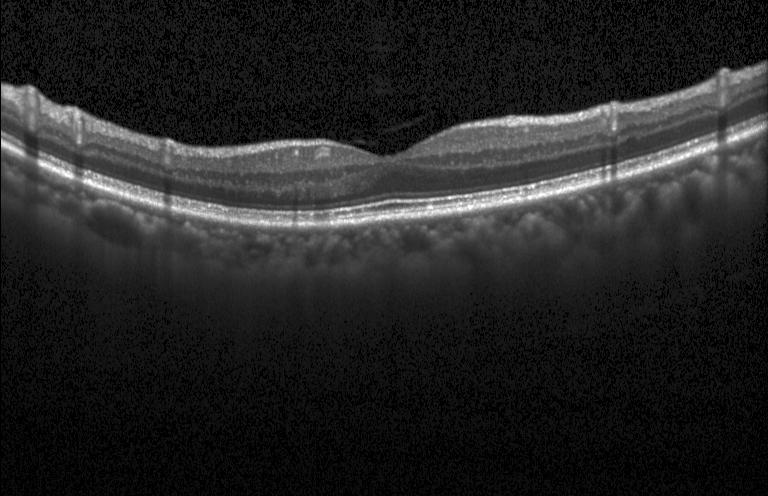
Finding: no evidence of CNV, DME, or drusen.